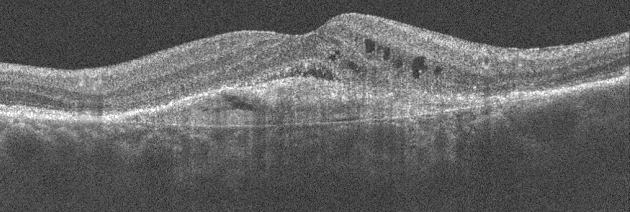 OS · optical coherence tomography B-scan.
Impression: age-related macular degeneration.